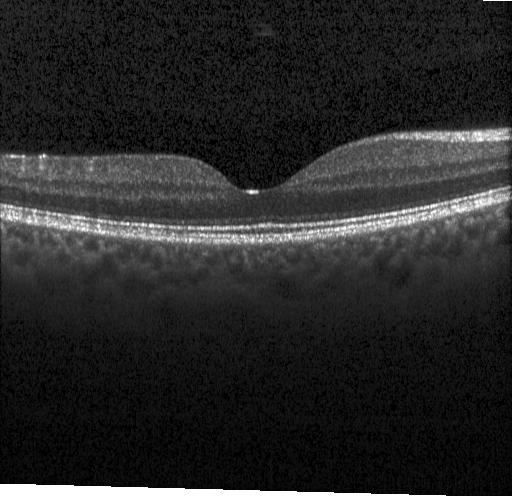
The scan shows neither choroidal neovascularization, diabetic macular edema, nor drusen.